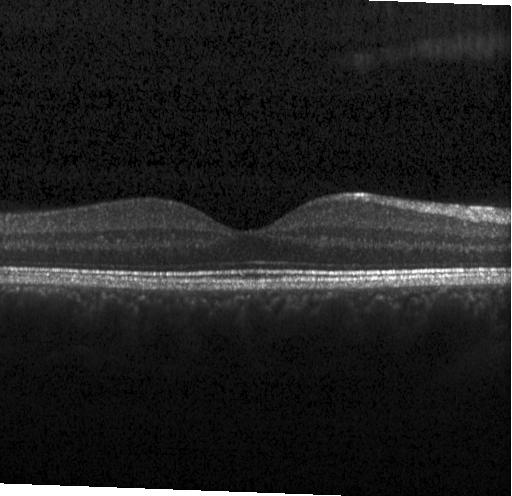

OCT finding: no evidence of CNV, DME, or drusen.